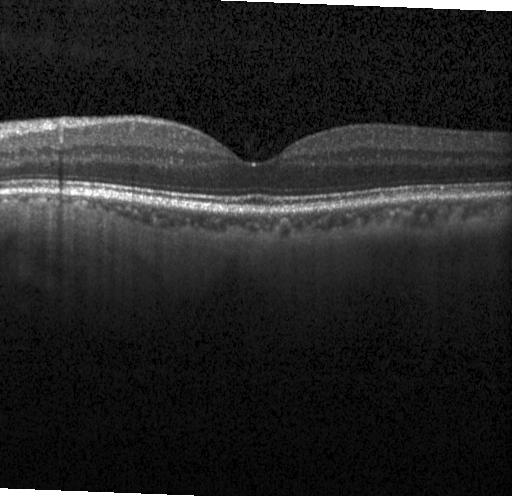

OCT B-scan. Spectral-domain optical coherence tomography. Acquired on a Heidelberg Spectralis. Assessment: no choroidal neovascularization, no diabetic macular edema, and no drusen.